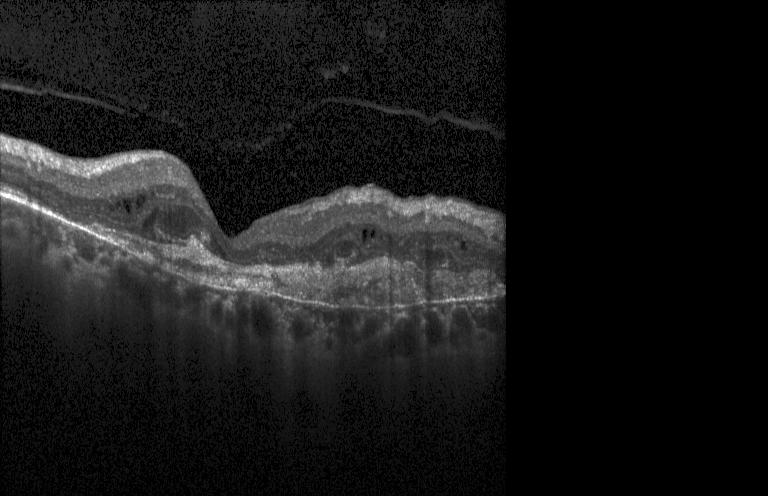
Optical coherence tomography scan; SD-OCT.
This B-scan demonstrates a choroidal neovascular membrane.